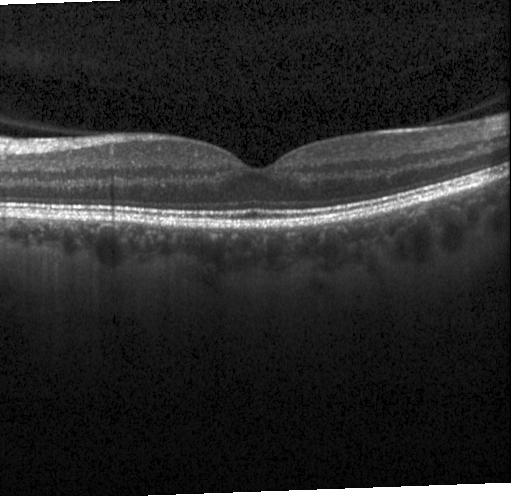
Assessment: neither CNV, DME, nor drusen.